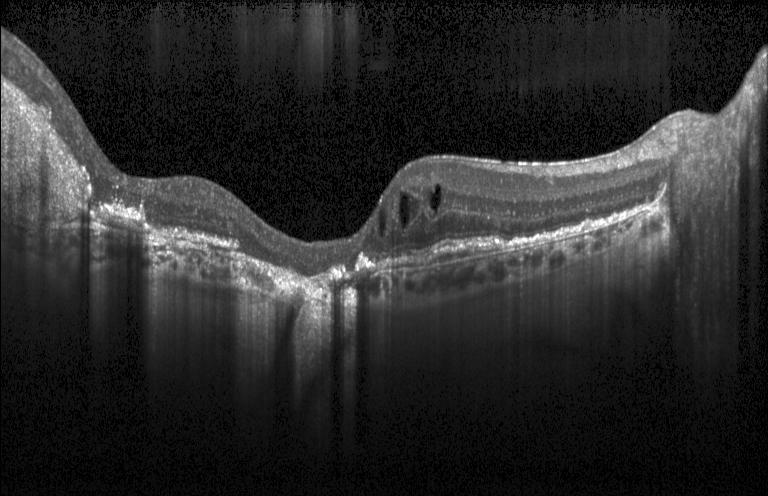

Centered on the fovea. Instrument: Heidelberg Spectralis. OCT B-scan. SD-OCT
Diagnosis: a choroidal neovascular membrane.